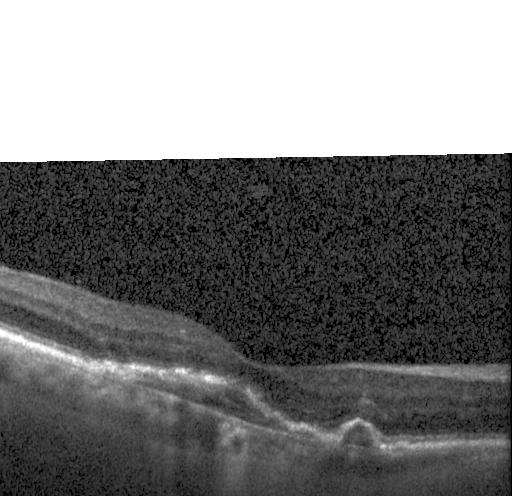 Horizontal scan through the fovea · acquired on a Heidelberg Spectralis · optical coherence tomography scan — Diagnosis: CNV.